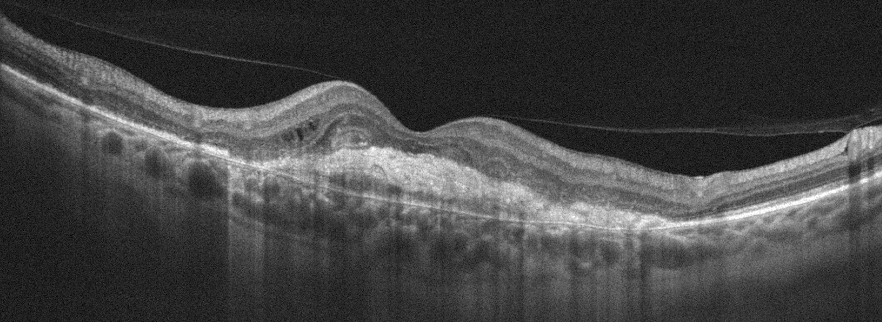 Right eye; instrument: Optovue Avanti RTVue XR; optical coherence tomography B-scan
The scan shows age-related macular degeneration (AMD).